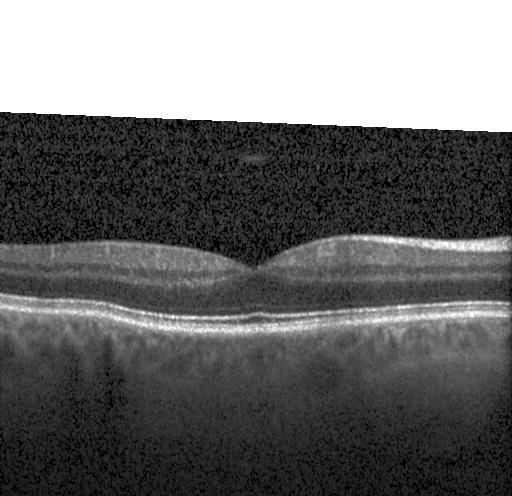

Assessment: no choroidal neovascularization, no diabetic macular edema, and no drusen.